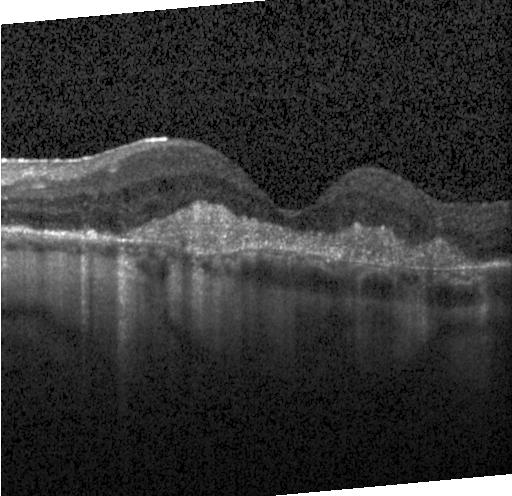
Horizontal scan through the fovea. Retinal OCT cross-section — This B-scan demonstrates choroidal neovascularization.